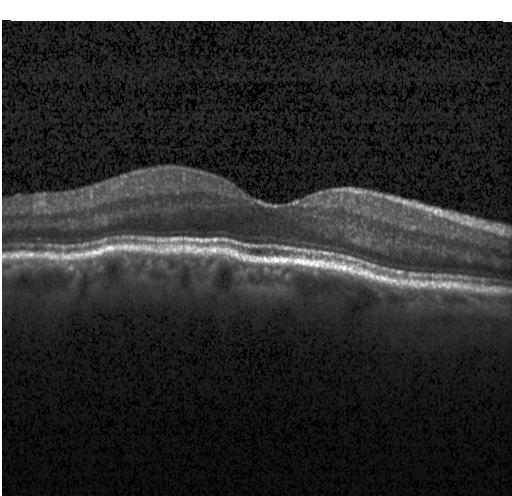
Heidelberg Spectralis OCT system; OCT line scan; spectral-domain optical coherence tomography.
Diagnosis: no CNV, no DME, and no drusen.